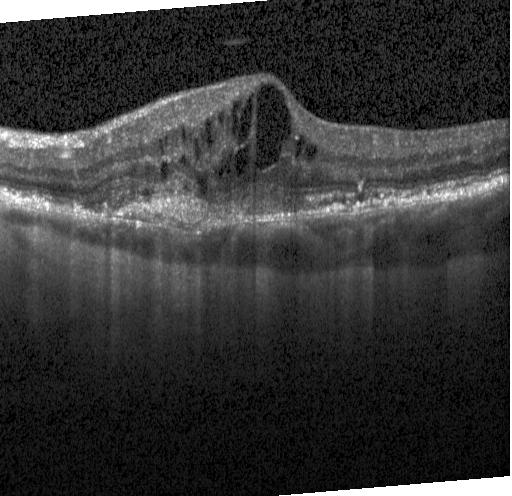 Finding: a choroidal neovascular membrane.